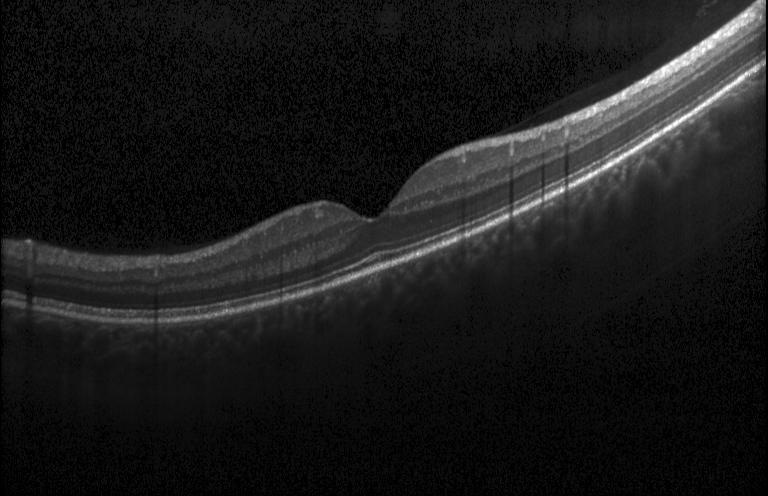

OCT line scan. Spectral-domain OCT. Impression: neither choroidal neovascularization, diabetic macular edema, nor drusen.